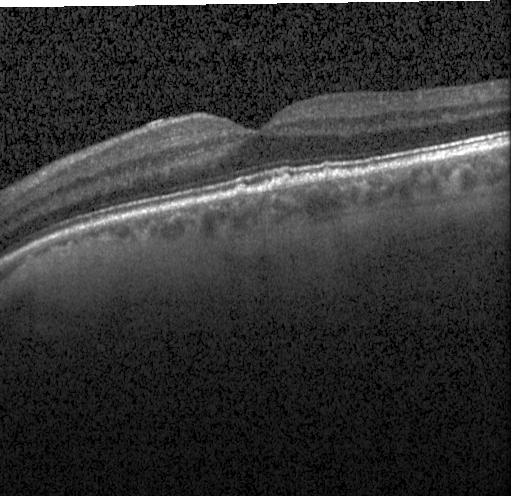 Spectral-domain optical coherence tomography, macular scan, optical coherence tomography B-scan. The scan shows multiple drusen.